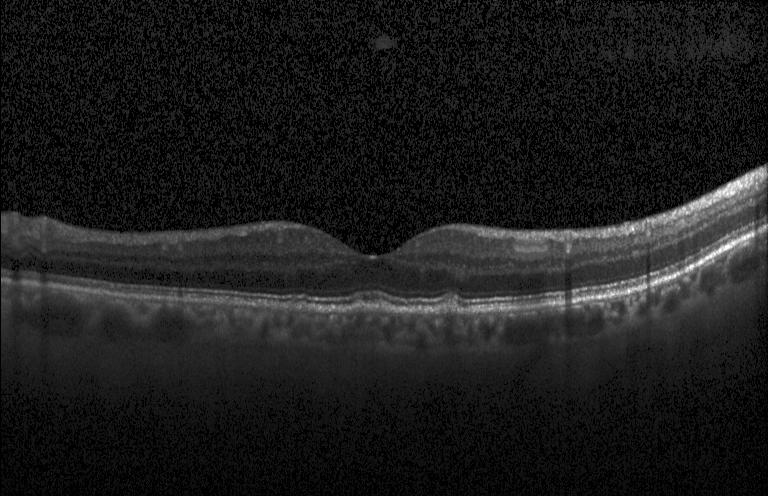 OCT B-scan · Heidelberg Spectralis · fovea-centered
OCT finding: multiple drusen.